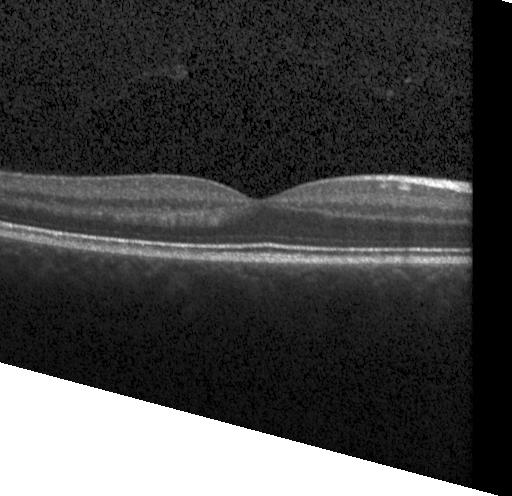

Fovea-centered; retinal OCT B-scan; spectral-domain optical coherence tomography; acquired on a Heidelberg Spectralis
Neither CNV, DME, nor drusen.